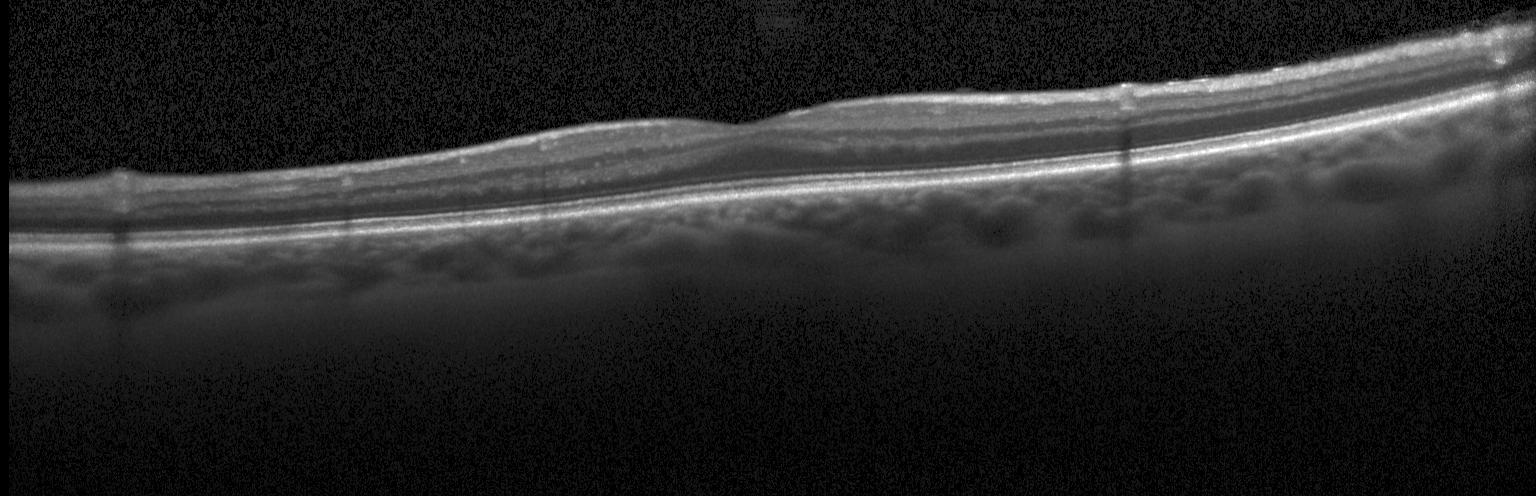

Macular OCT: no CNV, DME, or drusen.